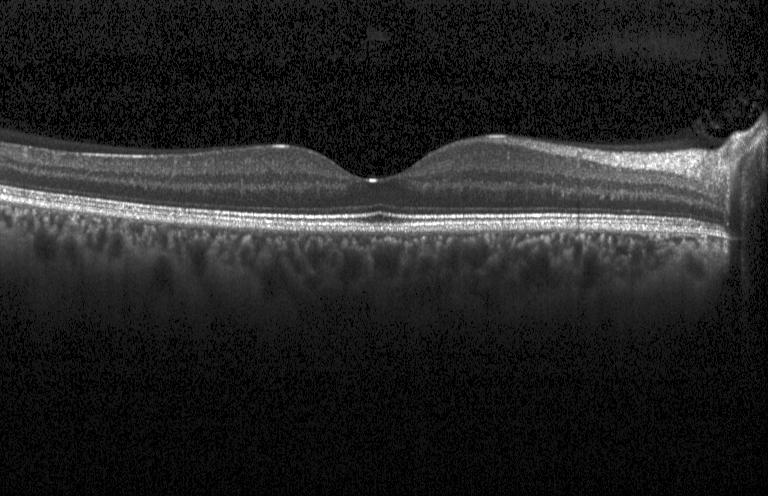

Dx: no choroidal neovascularization, no diabetic macular edema, and no drusen.